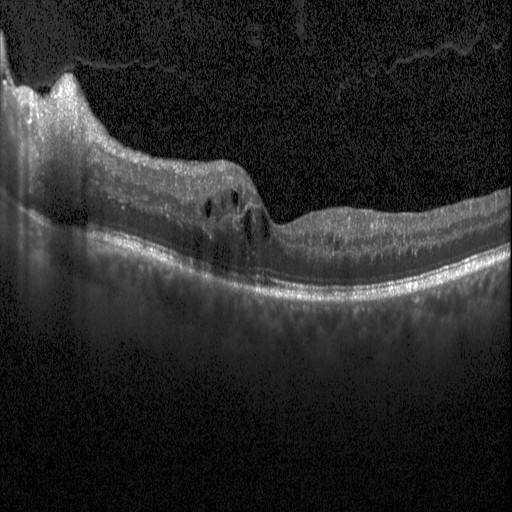
Optical coherence tomography B-scan.
Finding: diabetic macular edema.